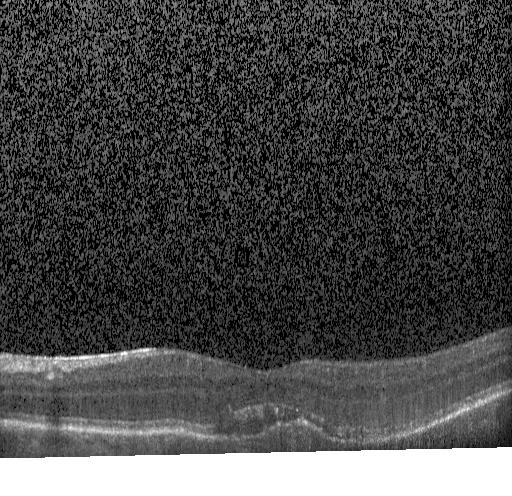
OCT line scan, spectral-domain OCT. The scan shows a choroidal neovascular membrane.